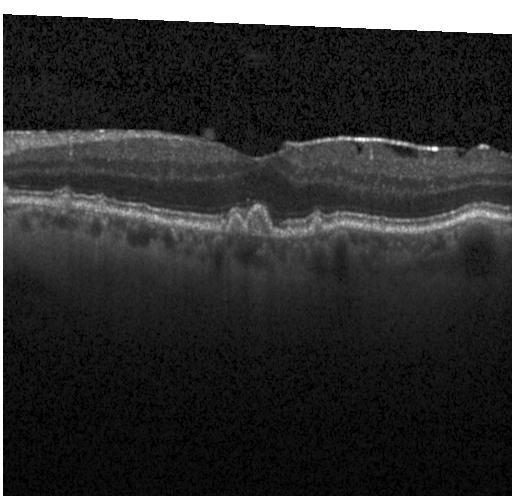
Dx: drusen.